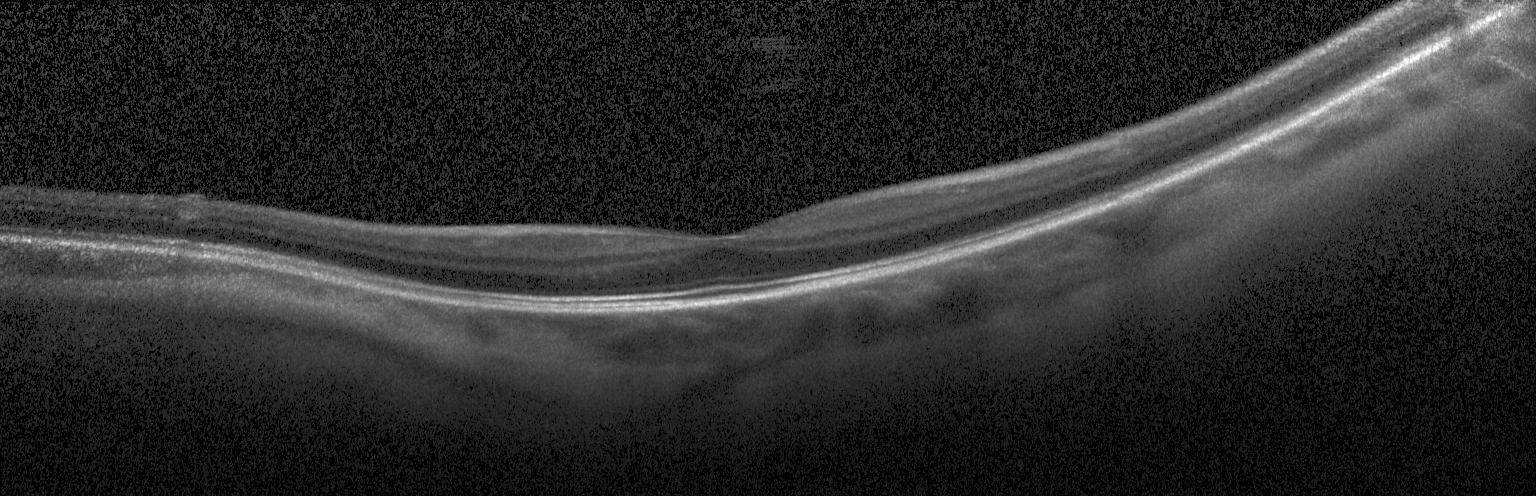
Impression: no choroidal neovascularization, diabetic macular edema, or drusen.